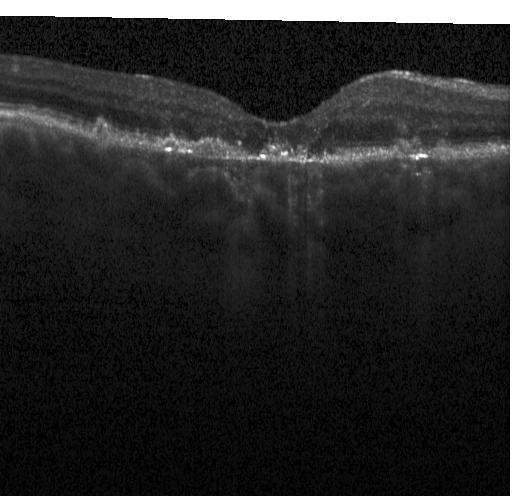

Spectral-domain optical coherence tomography · retinal OCT B-scan — Macular OCT: CNV.